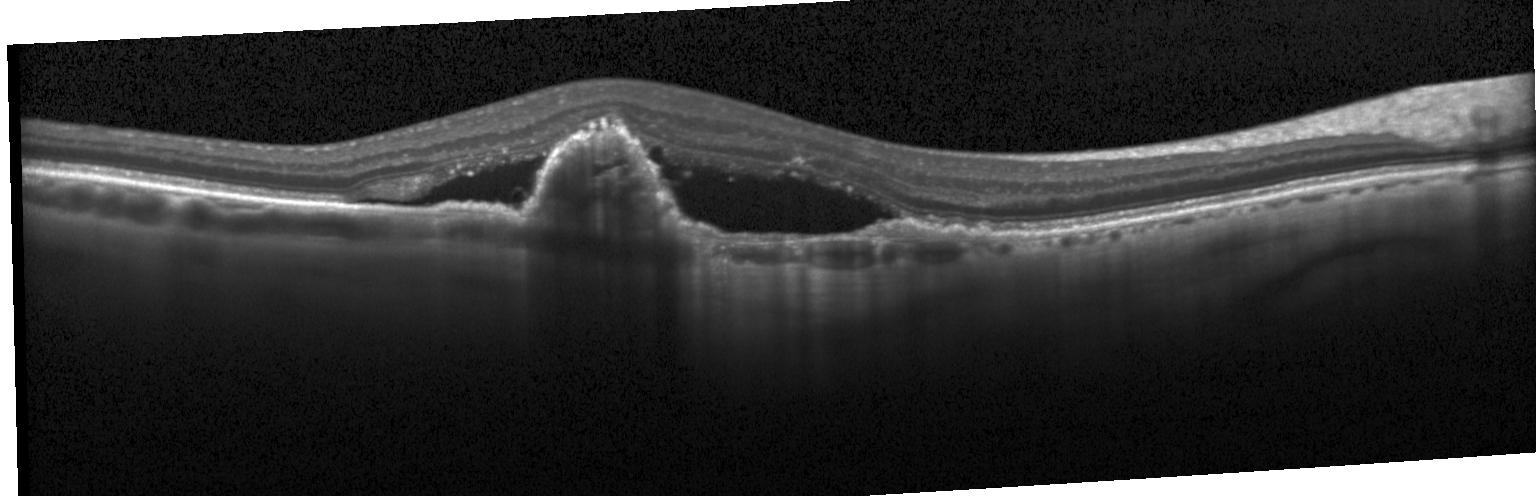

Spectral-domain OCT; centered on the fovea; Heidelberg Spectralis; OCT B-scan. Impression: a choroidal neovascular membrane.